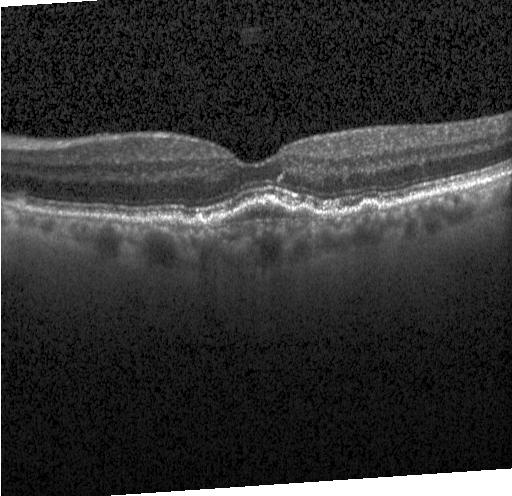
Spectral-domain optical coherence tomography; macular scan; Heidelberg Spectralis OCT system; OCT B-scan. Finding: choroidal neovascularization (CNV).